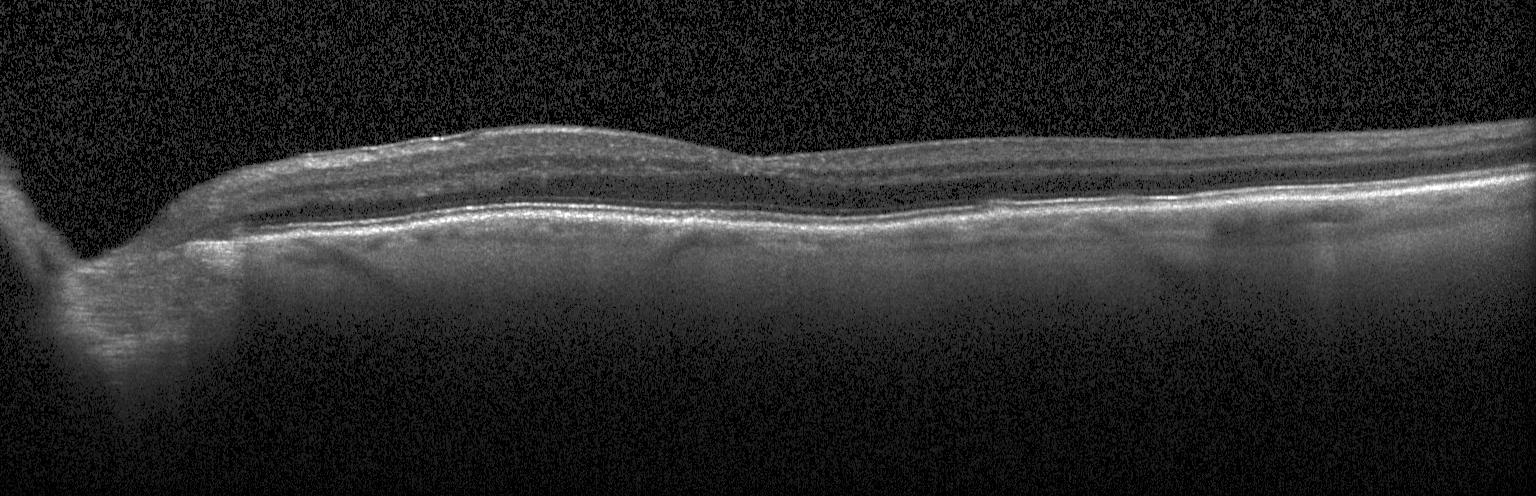 Horizontal scan through the fovea; optical coherence tomography scan; Heidelberg Spectralis; spectral-domain optical coherence tomography. Assessment: no evidence of choroidal neovascularization, diabetic macular edema, or drusen.